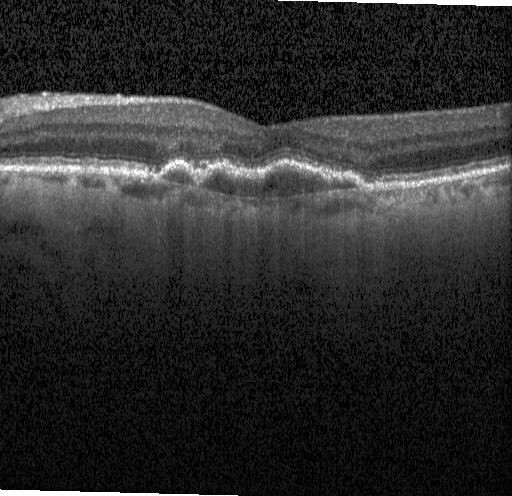
Through the macula. Optical coherence tomography B-scan — Finding: a choroidal neovascular membrane.